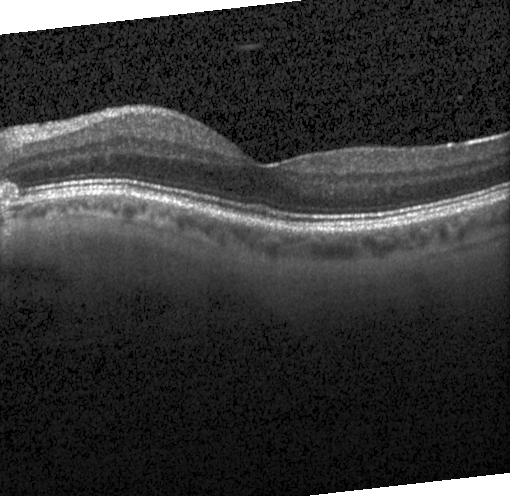

Spectral-domain OCT · macular scan · retinal OCT B-scan · instrument: Heidelberg Spectralis.
Diagnosis: drusen.